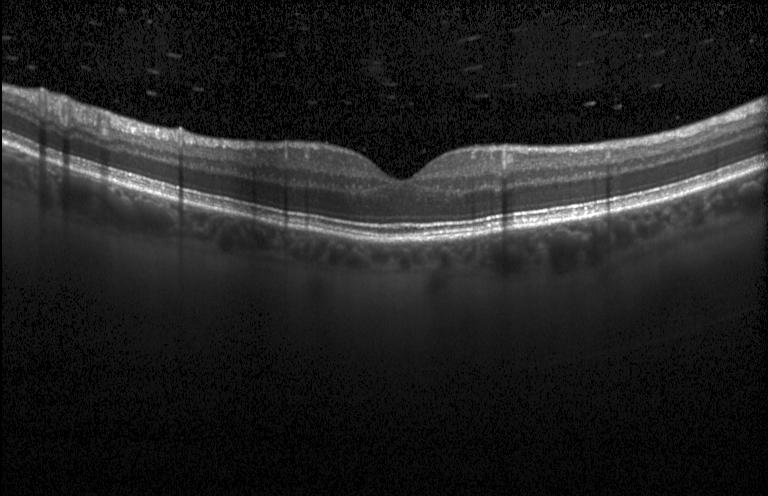 Retinal OCT cross-section showing no choroidal neovascularization, no diabetic macular edema, and no drusen.